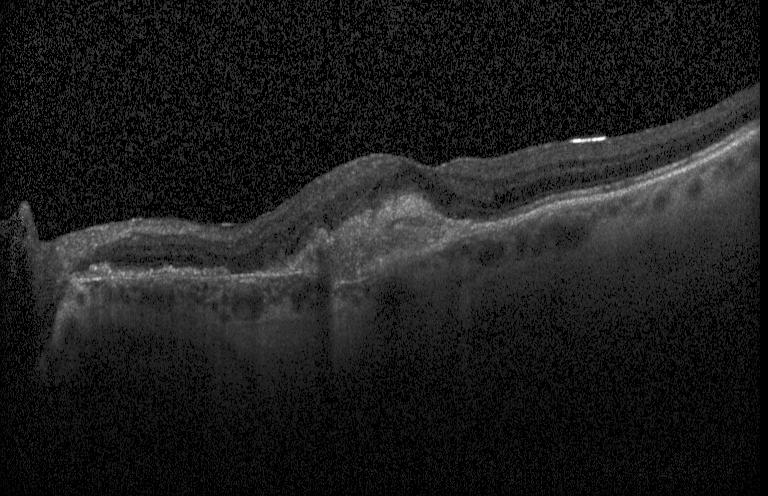

Impression: choroidal neovascularization (CNV).